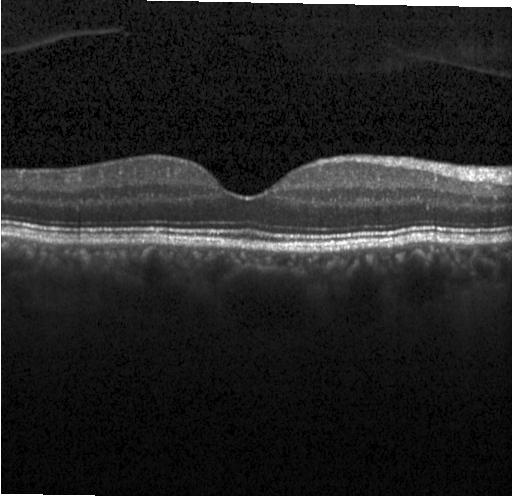
Diagnosis: no choroidal neovascularization, diabetic macular edema, or drusen.